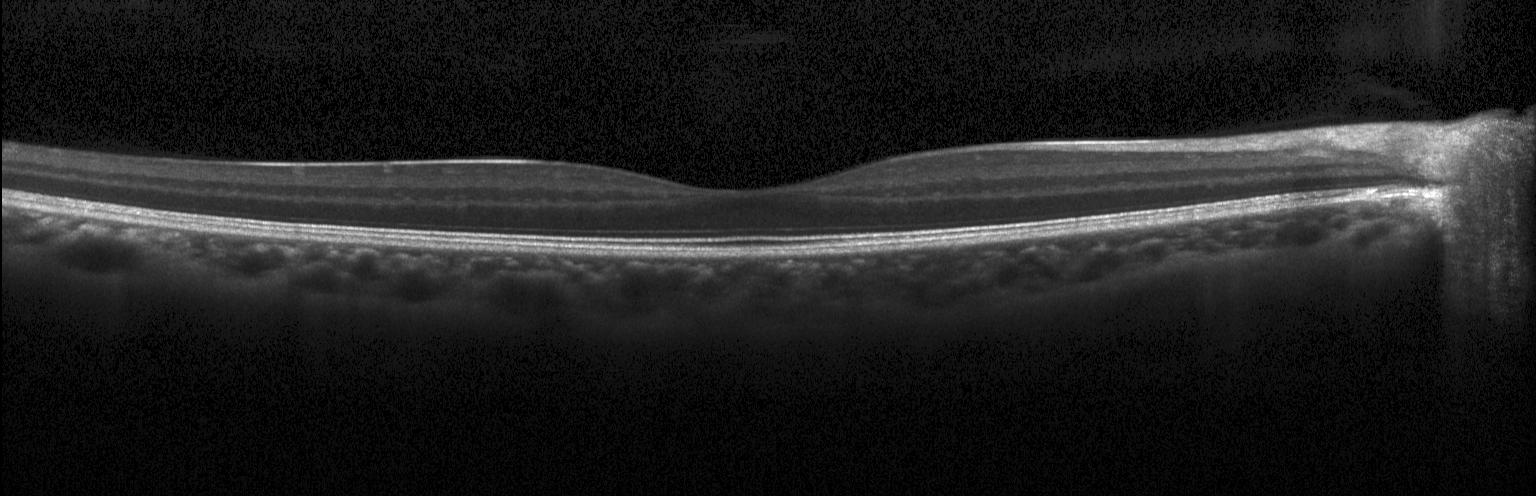

OCT line scan
This B-scan demonstrates neither choroidal neovascularization, diabetic macular edema, nor drusen.